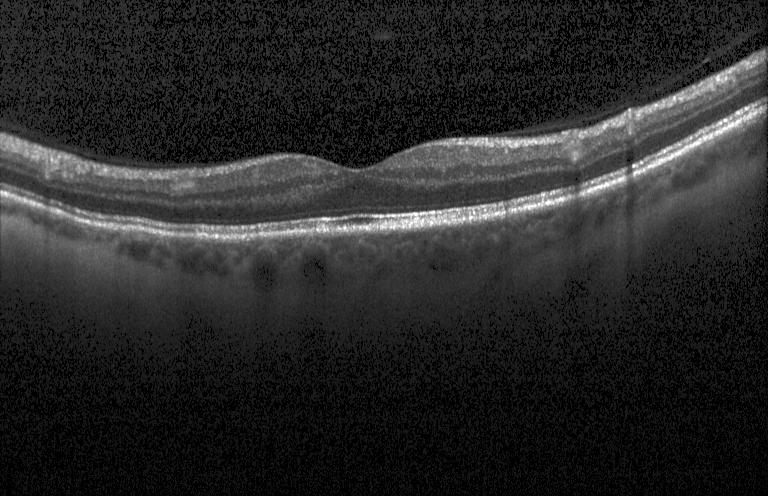
Impression: no CNV, DME, or drusen.